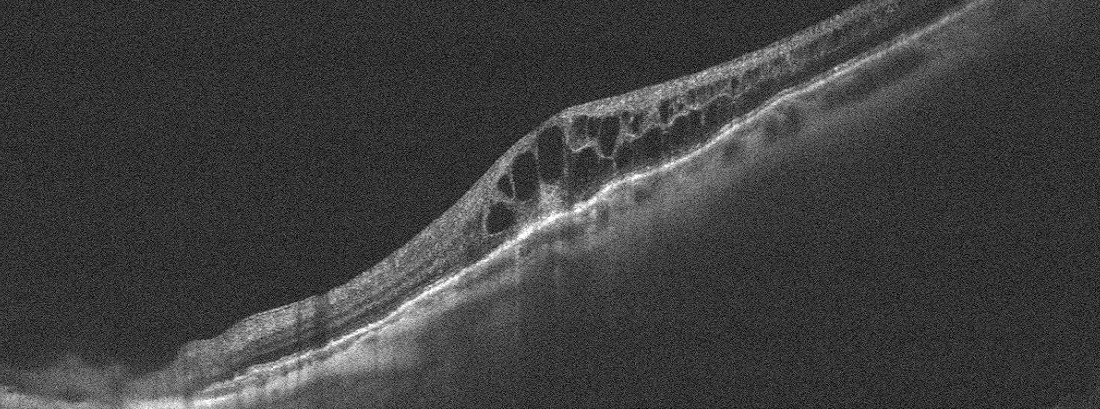

OCT B-scan
Diagnosis: RVO.